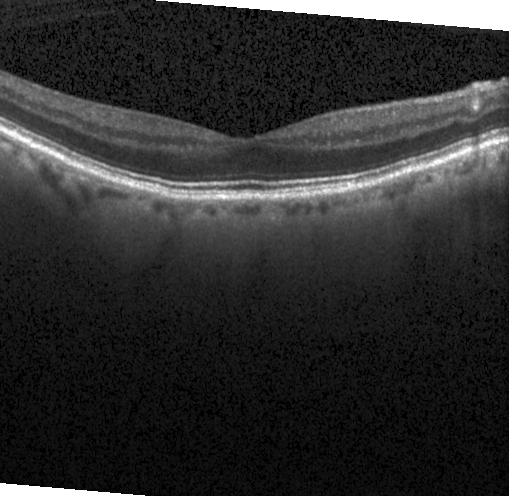
OCT B-scan · acquired on a Heidelberg Spectralis
Diagnosis: neither CNV, DME, nor drusen.